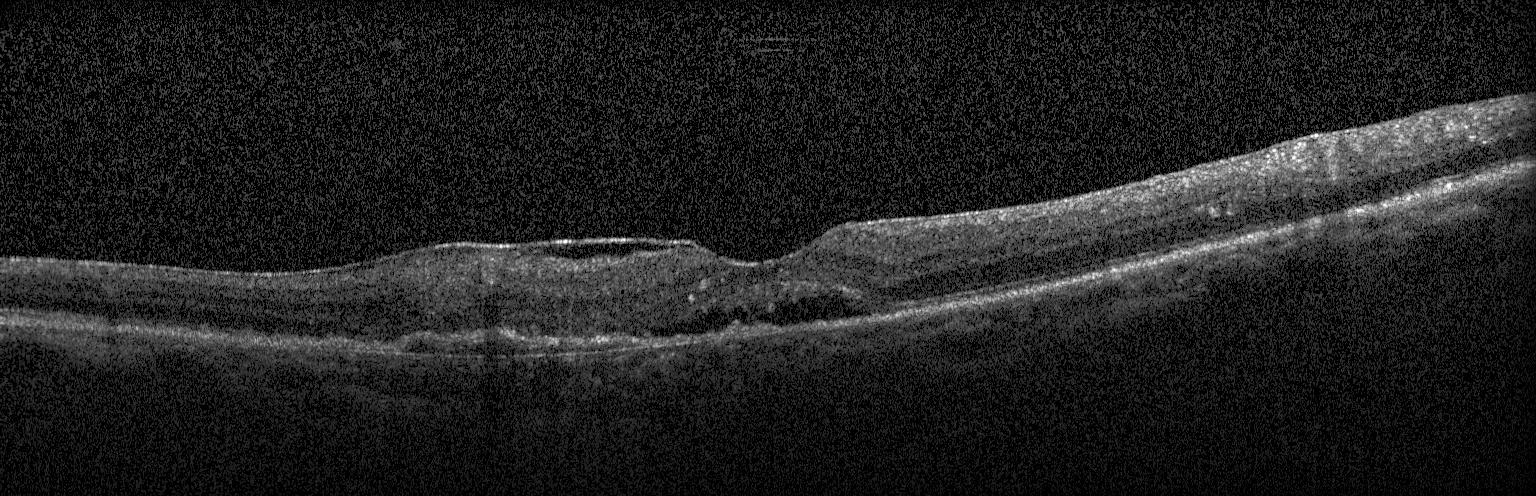 OCT finding: a choroidal neovascular membrane.